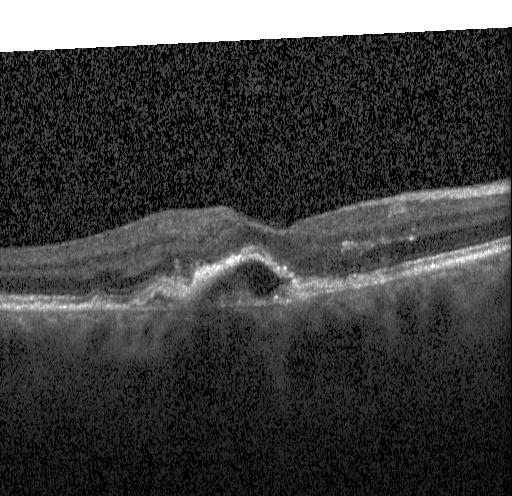
Heidelberg Spectralis OCT system; OCT line scan; horizontal scan through the fovea. Finding: a choroidal neovascular membrane.